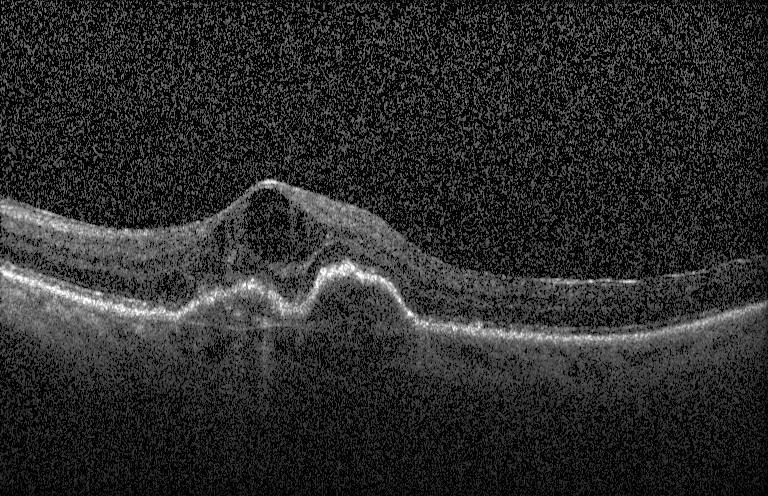 OCT finding: choroidal neovascularization.